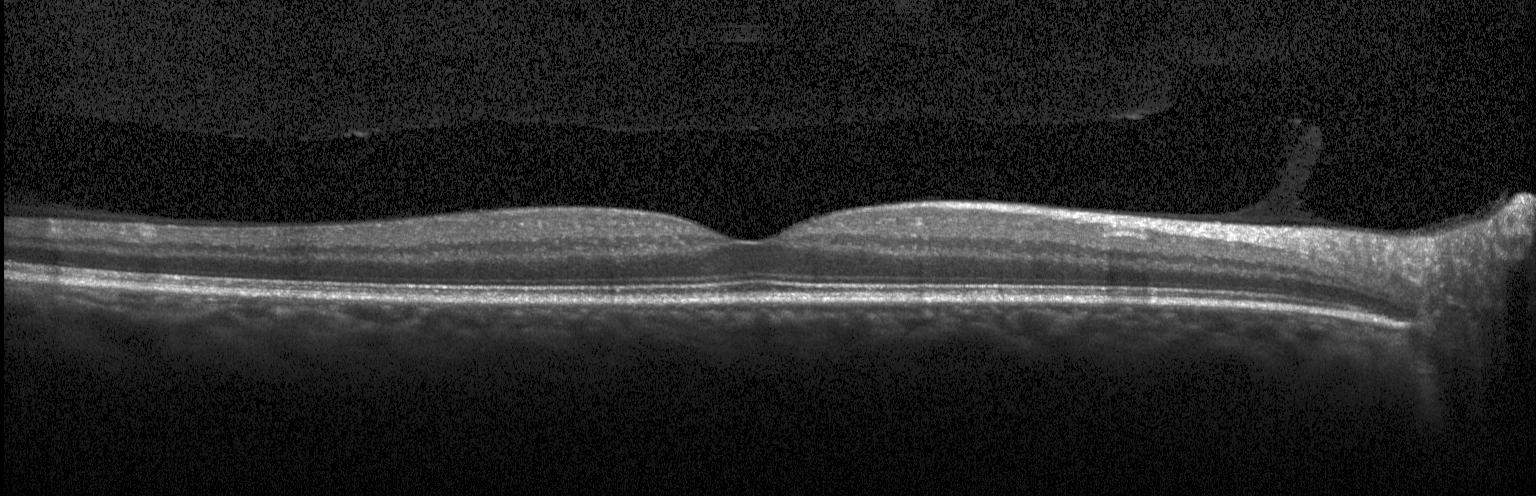
Spectral-domain OCT; Heidelberg Spectralis OCT system; OCT line scan.
This B-scan demonstrates neither choroidal neovascularization, diabetic macular edema, nor drusen.